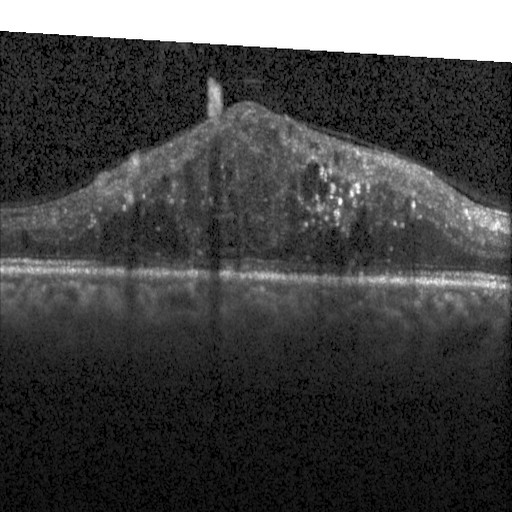

Spectral-domain OCT · retinal OCT cross-section. Impression: diabetic macular edema (DME).